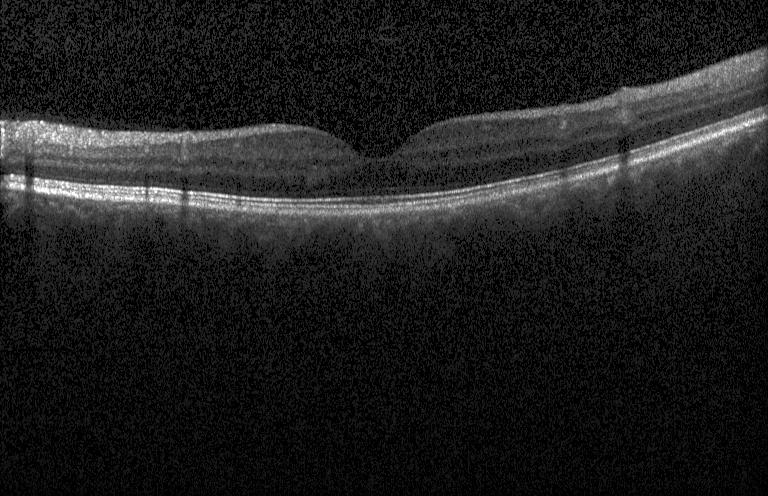

Through the macula. Instrument: Heidelberg Spectralis. OCT line scan
Impression: neither choroidal neovascularization, diabetic macular edema, nor drusen.